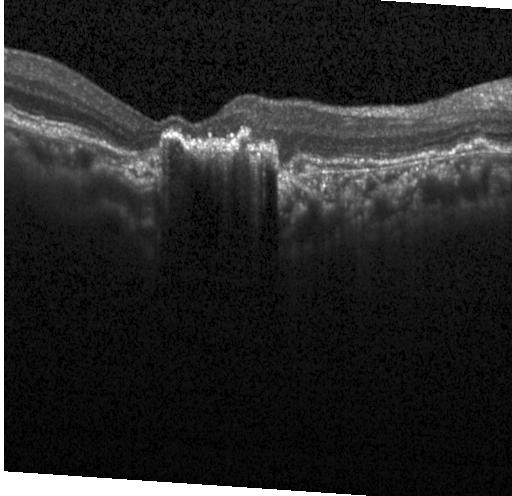

Spectral-domain OCT; acquired on a Heidelberg Spectralis; retinal OCT B-scan
The scan shows a choroidal neovascular membrane.